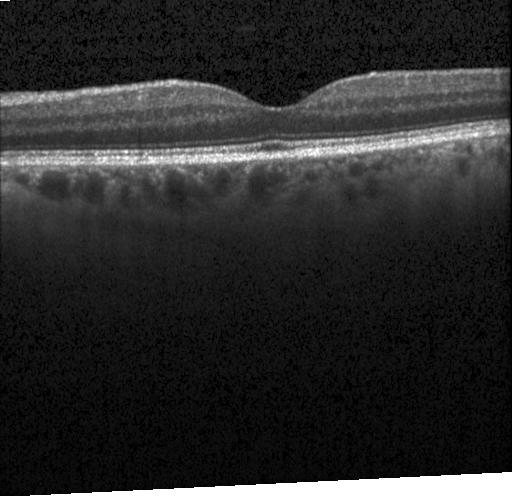 OCT finding: no CNV, no DME, and no drusen.